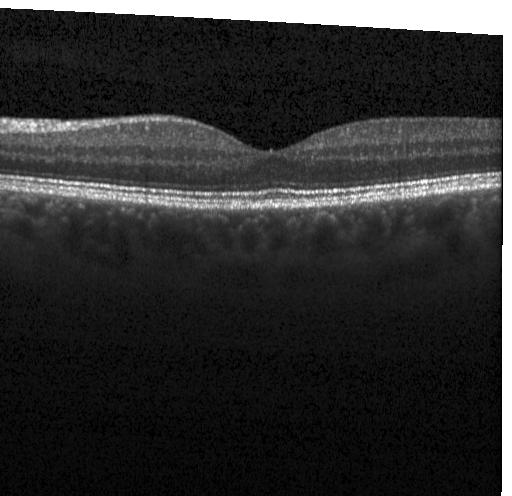 Optical coherence tomography scan — Finding: no choroidal neovascularization, diabetic macular edema, or drusen.